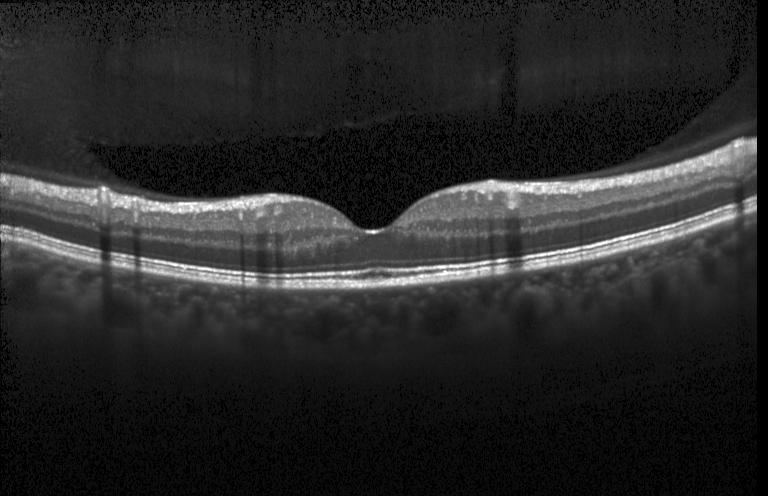 Spectral-domain optical coherence tomography. Macular scan. Retinal OCT cross-section. Heidelberg Spectralis OCT system
Diagnosis: no choroidal neovascularization, diabetic macular edema, or drusen.